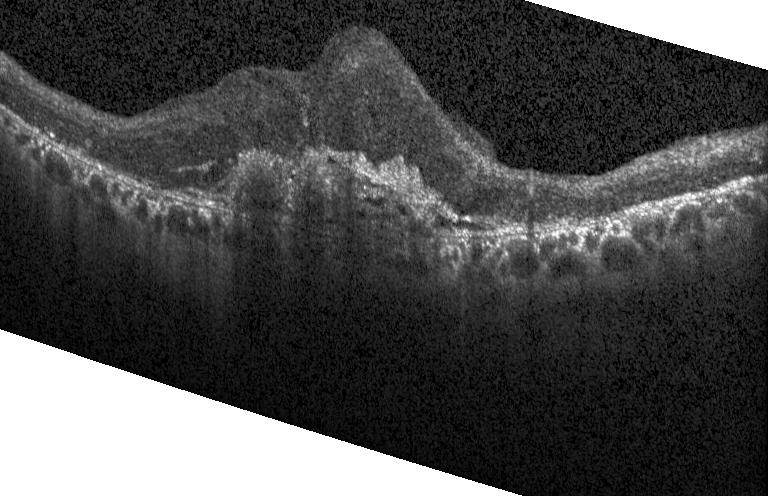 Optical coherence tomography scan, Heidelberg Spectralis OCT system, macular scan. This B-scan demonstrates CNV.